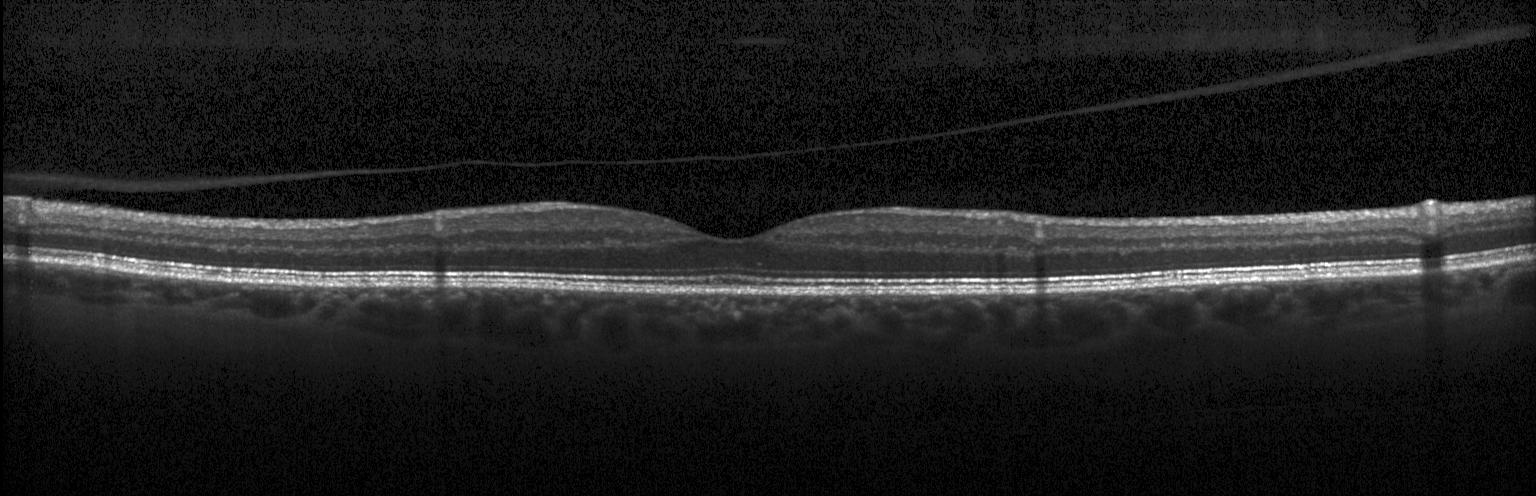

Retinal OCT cross-section showing no evidence of choroidal neovascularization, diabetic macular edema, or drusen.